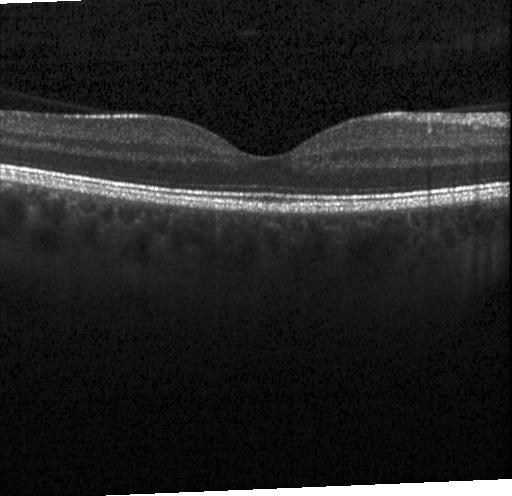
Macular OCT demonstrating no evidence of CNV, DME, or drusen.